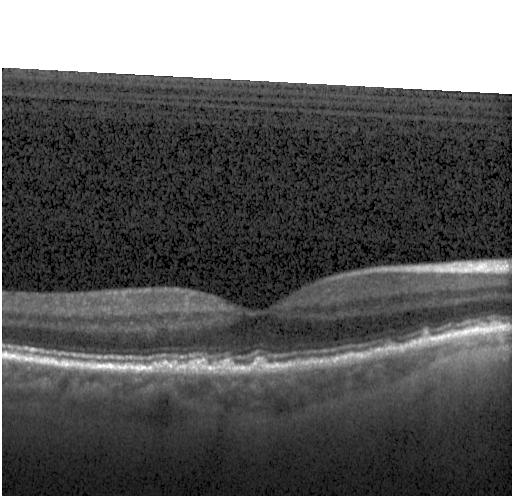
Heidelberg Spectralis · OCT line scan. The scan shows sub-RPE drusenoid deposits.